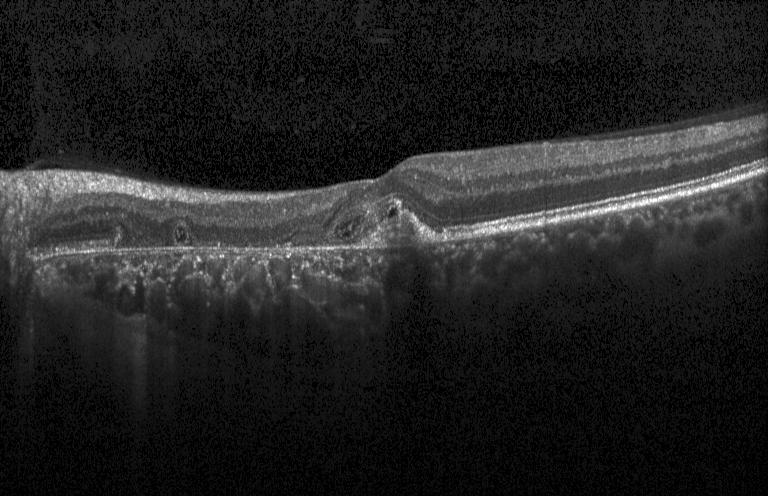 Impression: a choroidal neovascular membrane.